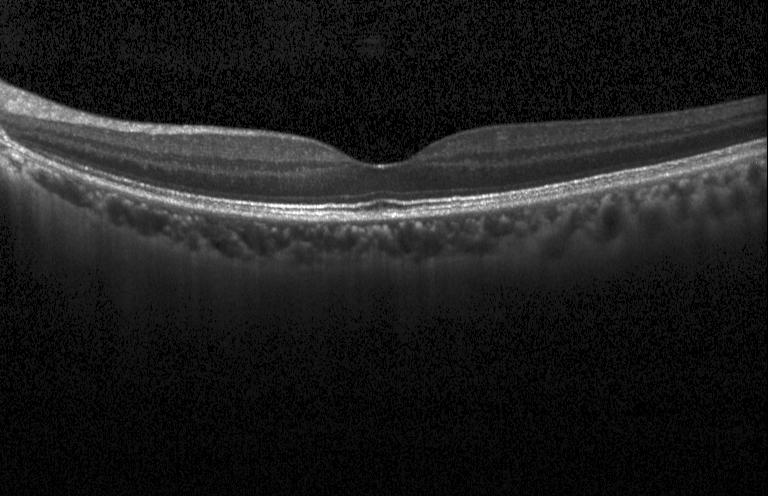 Finding: no choroidal neovascularization, diabetic macular edema, or drusen.